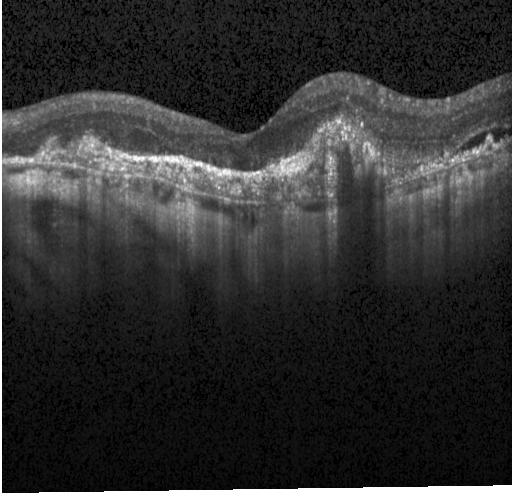

SD-OCT. Horizontal scan through the fovea. Optical coherence tomography scan. Heidelberg Spectralis
Finding: CNV.